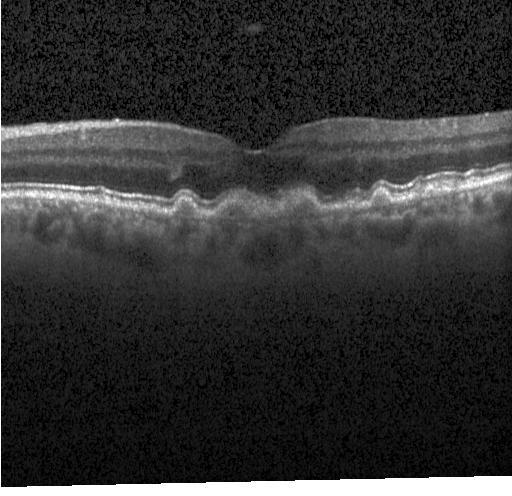
Impression: drusen.